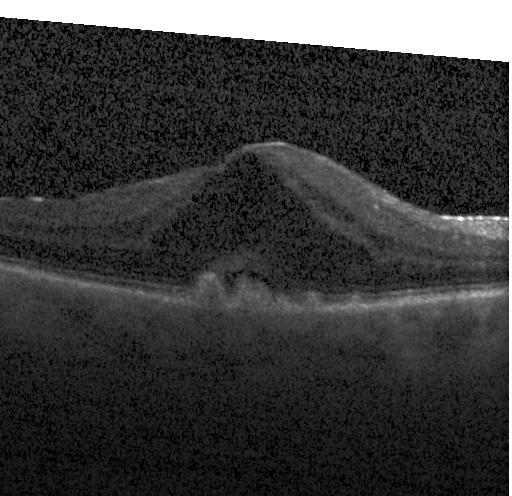
Through the macula; OCT B-scan.
Finding: choroidal neovascularization.